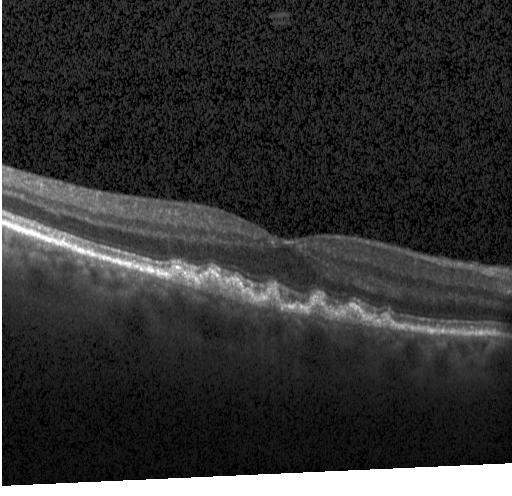

SD-OCT; Heidelberg Spectralis; OCT B-scan.
This B-scan demonstrates multiple drusen.